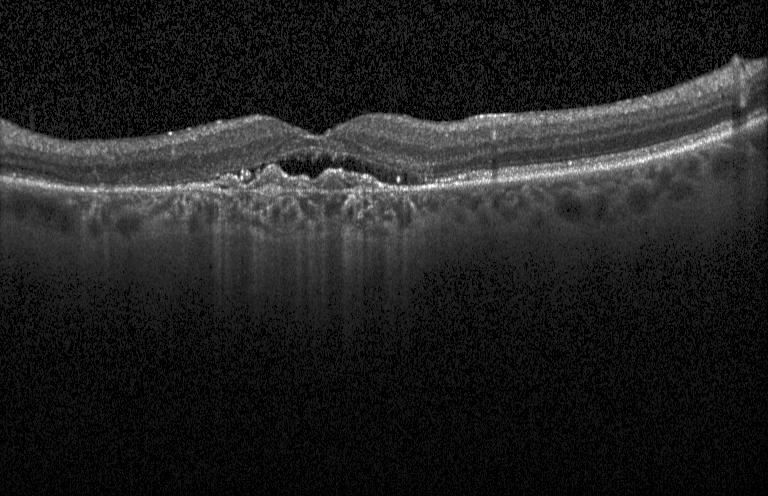
Fovea-centered · spectral-domain OCT · optical coherence tomography scan
Macular OCT: a choroidal neovascular membrane.